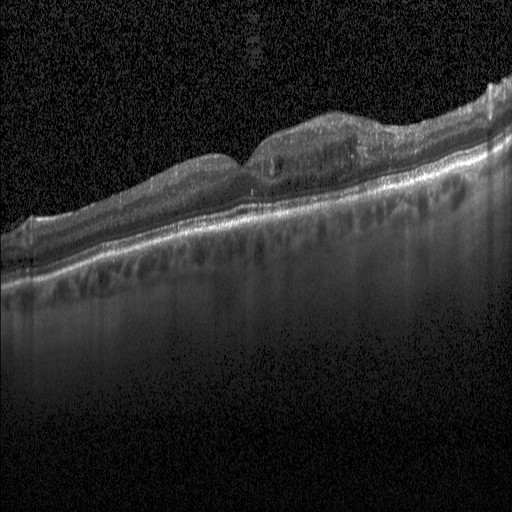

Optical coherence tomography B-scan — Diagnosis: diabetic macular edema.